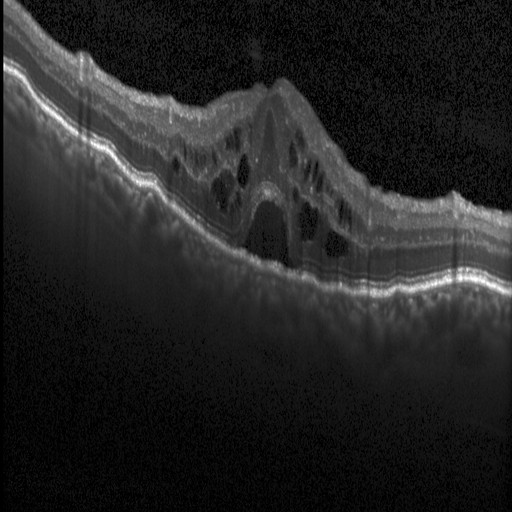 Optical coherence tomography scan
The scan shows diabetic macular edema.